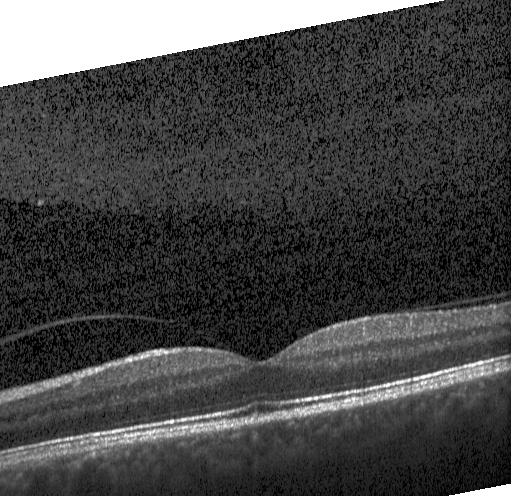

Optical coherence tomography B-scan · instrument: Heidelberg Spectralis. Dx: no choroidal neovascularization, diabetic macular edema, or drusen.